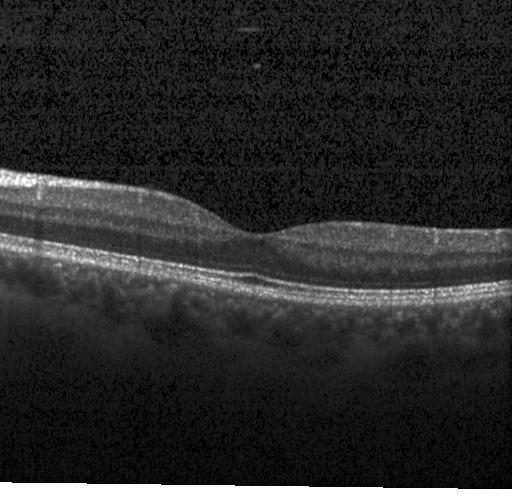

Centered on the fovea · acquired on a Heidelberg Spectralis · optical coherence tomography B-scan. Finding: no choroidal neovascularization, no diabetic macular edema, and no drusen.